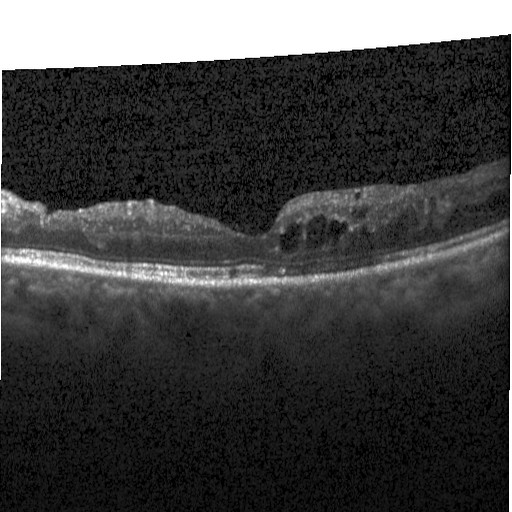
Retinal OCT cross-section. Assessment: diabetic macular edema.